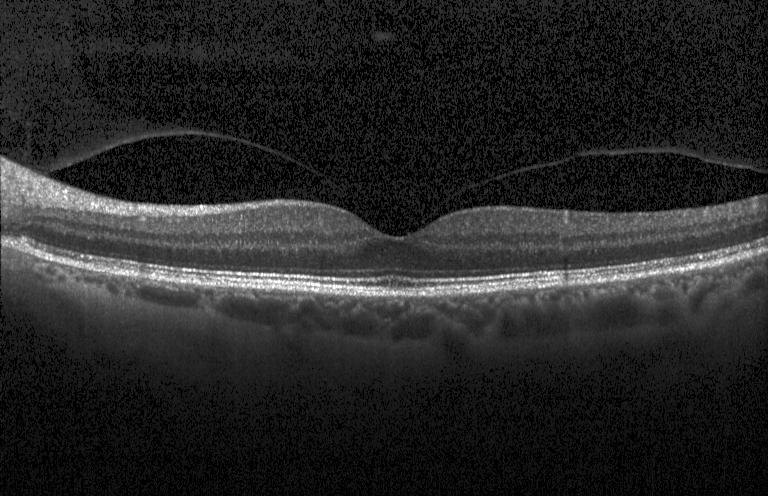

OCT B-scan · SD-OCT. Diagnosis: no choroidal neovascularization, no diabetic macular edema, and no drusen.